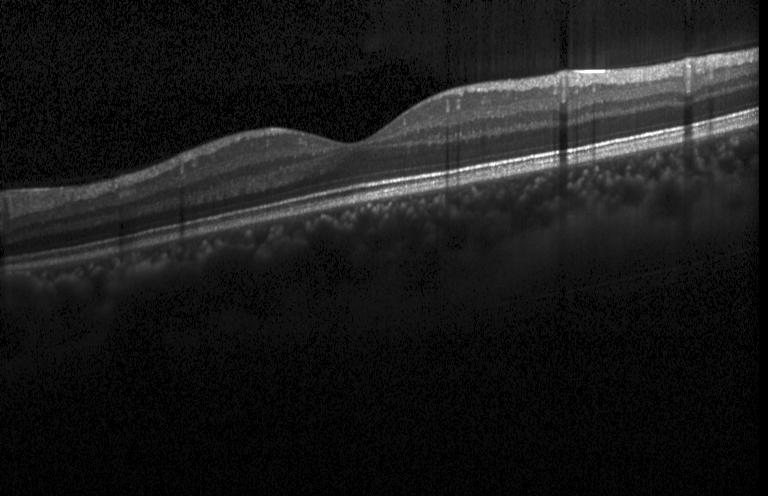
Retinal OCT cross-section · instrument: Heidelberg Spectralis · SD-OCT · fovea-centered
Diagnosis: no CNV, no DME, and no drusen.